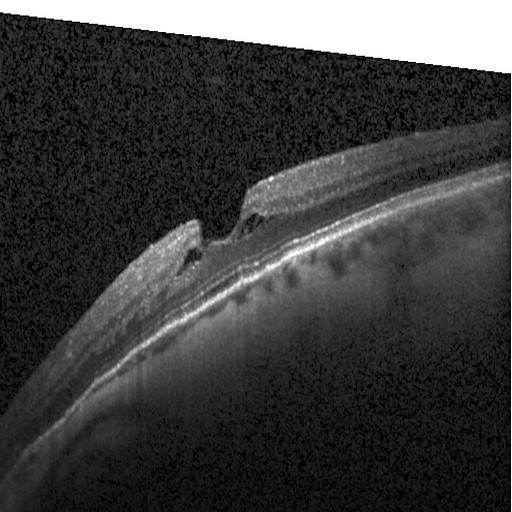

OCT B-scan · SD-OCT · horizontal scan through the fovea · acquired on a Heidelberg Spectralis.
The scan shows DME.